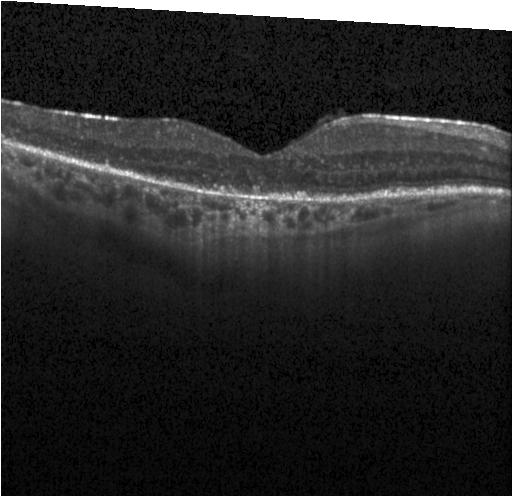
OCT B-scan · macular scan · spectral-domain optical coherence tomography · acquired on a Heidelberg Spectralis
Diagnosis: neither choroidal neovascularization, diabetic macular edema, nor drusen.